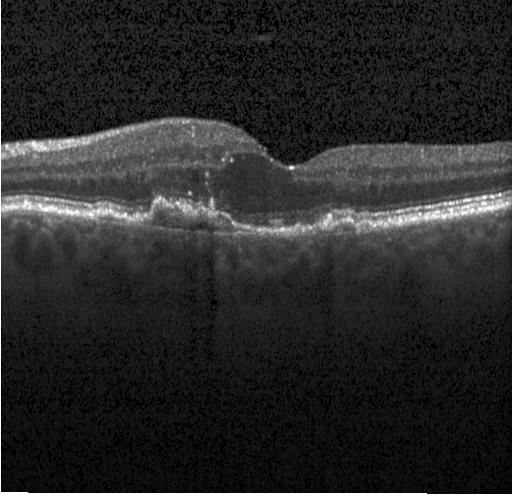 Fovea-centered. SD-OCT. OCT B-scan — Impression: choroidal neovascularization (CNV).